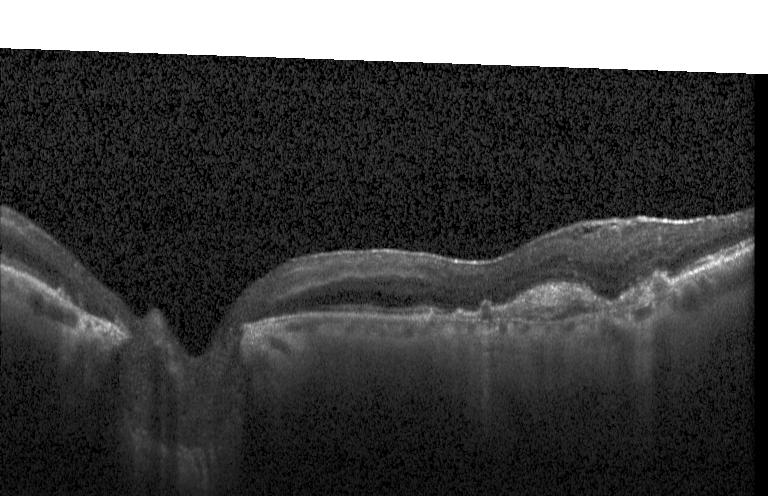
Heidelberg Spectralis, spectral-domain optical coherence tomography, OCT B-scan, through the macula
Assessment: a choroidal neovascular membrane.